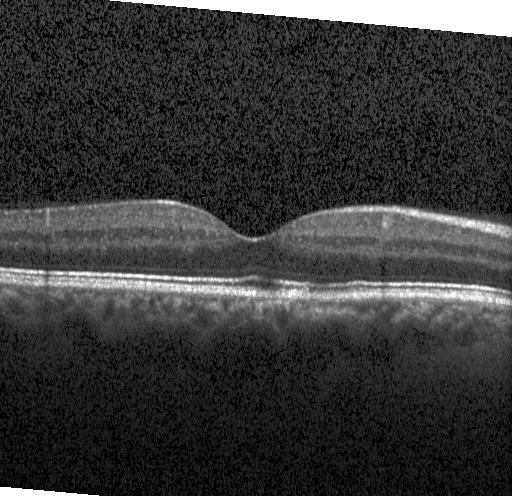 No choroidal neovascularization, no diabetic macular edema, and no drusen.